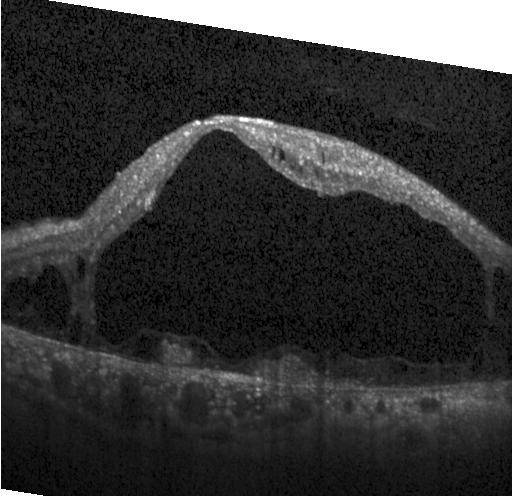 OCT finding: DME.